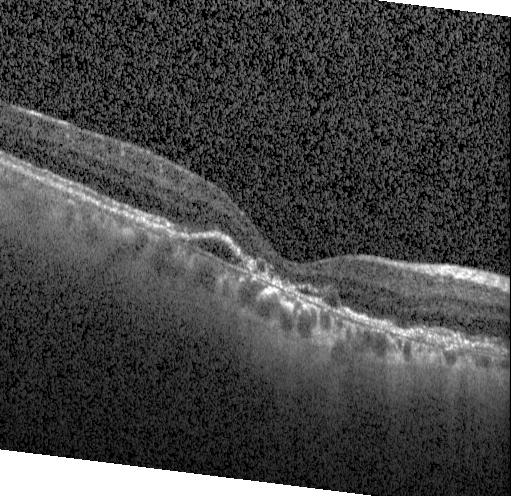

Macular OCT demonstrating a choroidal neovascular membrane.